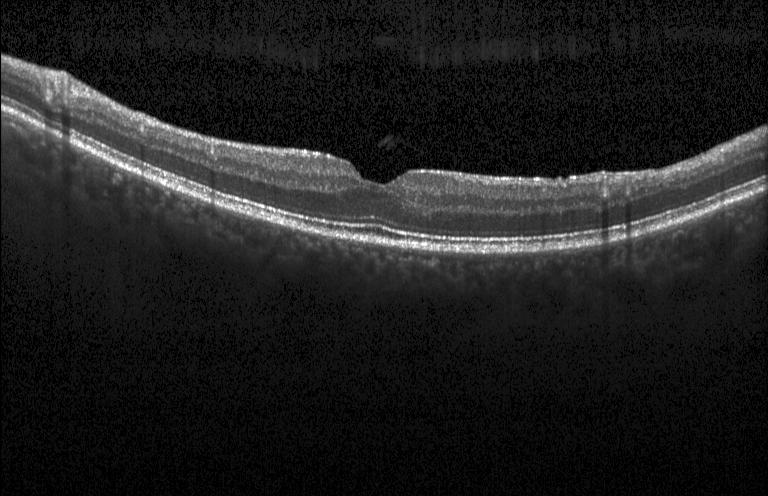

Spectral-domain optical coherence tomography, OCT B-scan, through the macula — Macular OCT: no CNV, DME, or drusen.